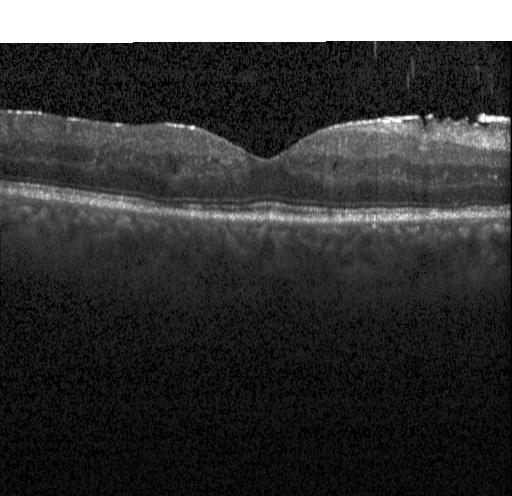 This B-scan demonstrates diabetic macular edema (DME).